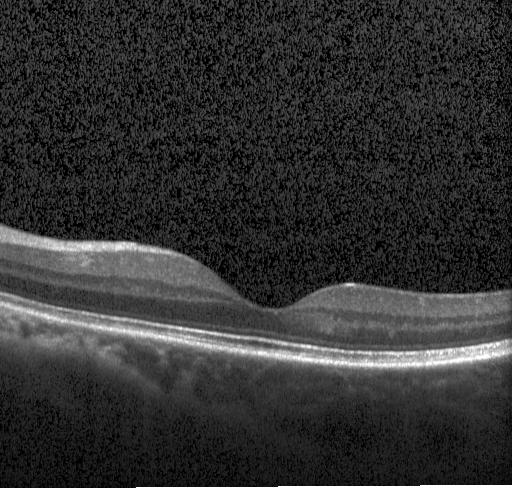
Retinal OCT B-scan
Diagnosis: no choroidal neovascularization, no diabetic macular edema, and no drusen.